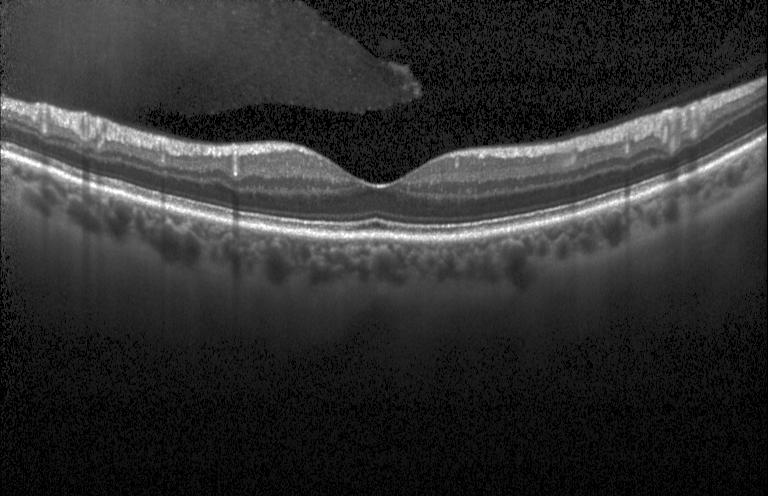
Optical coherence tomography scan; instrument: Heidelberg Spectralis
Dx: neither CNV, DME, nor drusen.